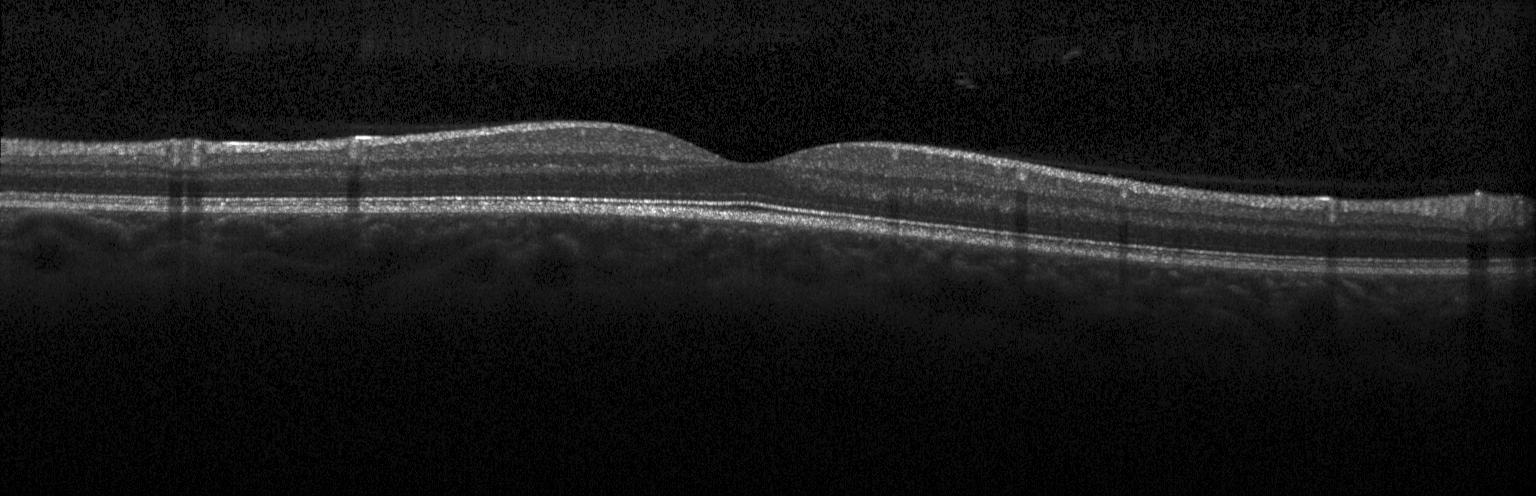 Retinal OCT B-scan · Heidelberg Spectralis OCT system · SD-OCT. Assessment: neither choroidal neovascularization, diabetic macular edema, nor drusen.